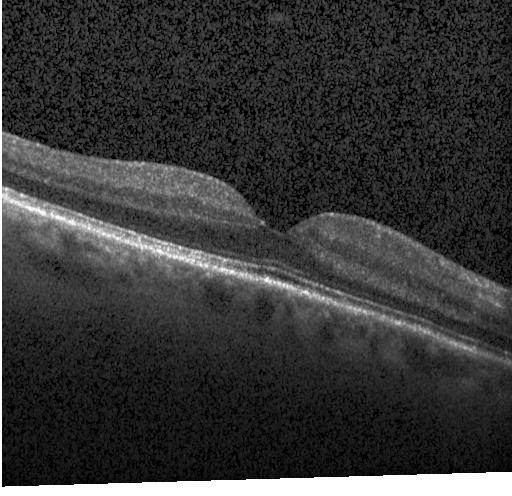
Assessment: no choroidal neovascularization, diabetic macular edema, or drusen.